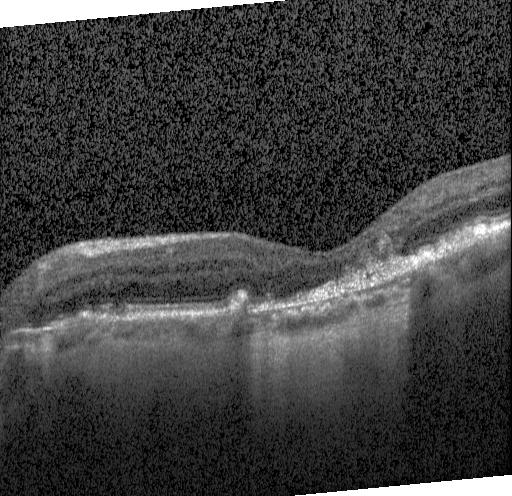 Spectral-domain OCT; centered on the fovea; optical coherence tomography B-scan.
Diagnosis: choroidal neovascularization (CNV).